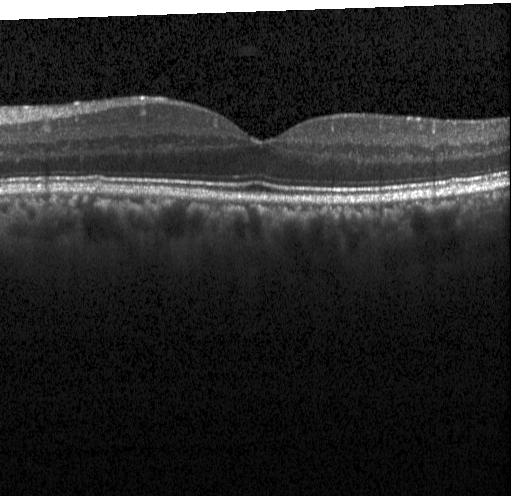

Acquired on a Heidelberg Spectralis · macular scan · optical coherence tomography scan · spectral-domain OCT. Drusen.